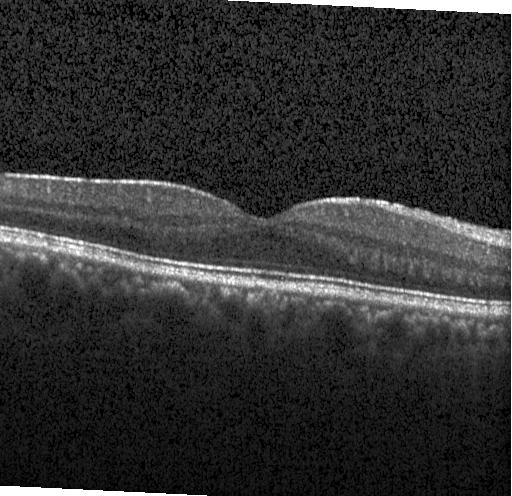

Heidelberg Spectralis OCT system. OCT line scan. Spectral-domain optical coherence tomography. The scan shows no evidence of choroidal neovascularization, diabetic macular edema, or drusen.